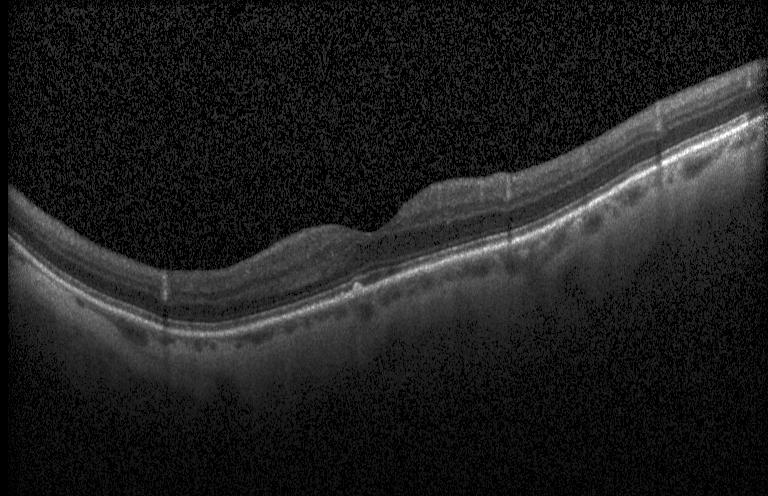

Spectral-domain optical coherence tomography, OCT B-scan, macular scan, acquired on a Heidelberg Spectralis.
Impression: drusen.